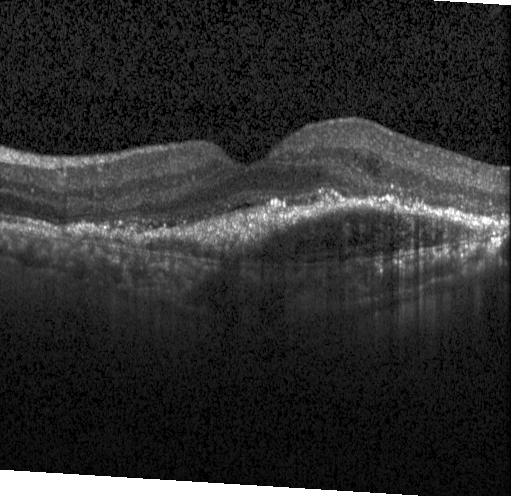

Acquired on a Heidelberg Spectralis, OCT line scan, macular scan. Macular OCT: CNV.